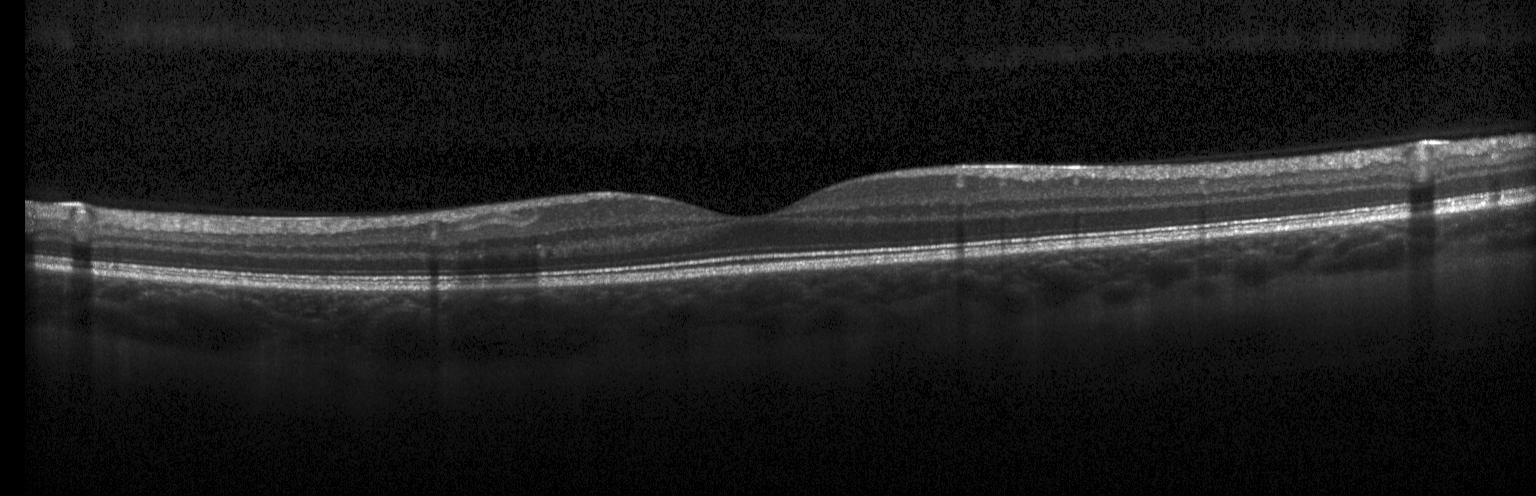 OCT B-scan; Heidelberg Spectralis OCT system.
OCT finding: neither choroidal neovascularization, diabetic macular edema, nor drusen.